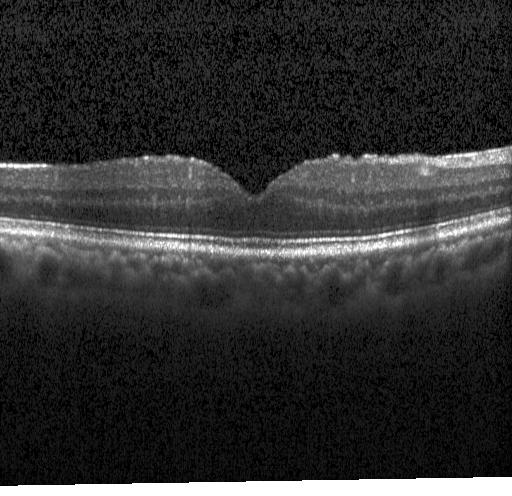 Diagnosis: no choroidal neovascularization, diabetic macular edema, or drusen.